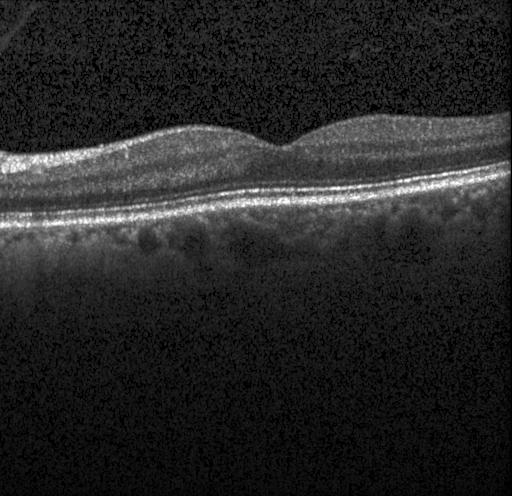 Horizontal scan through the fovea, retinal OCT cross-section. Dx: no choroidal neovascularization, diabetic macular edema, or drusen.